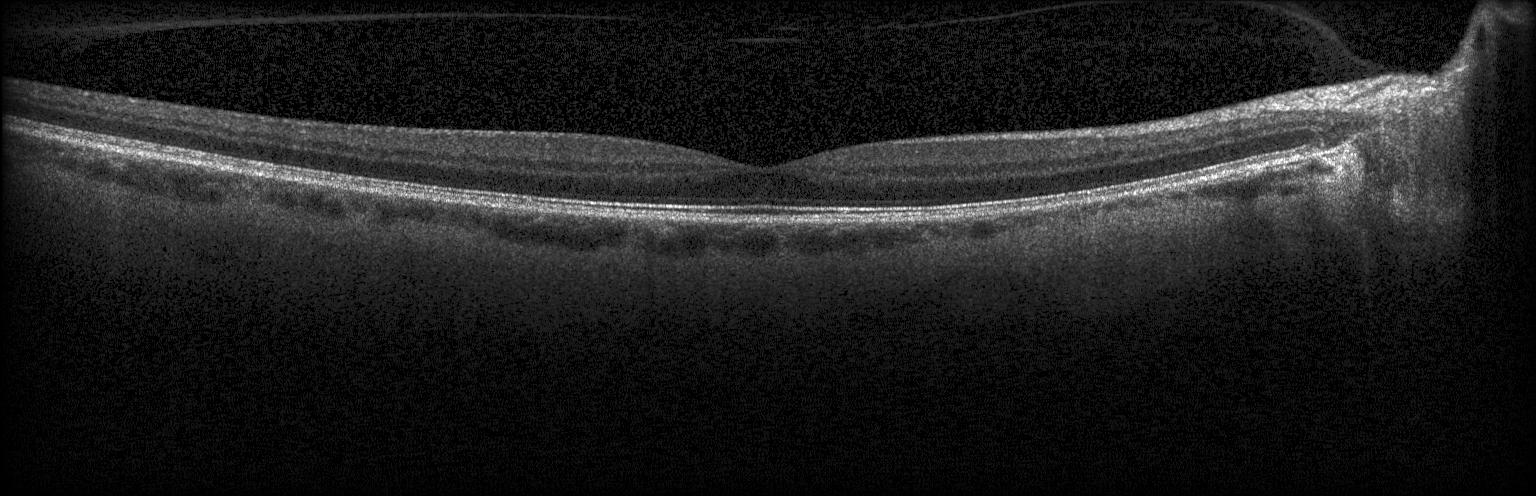 Horizontal scan through the fovea · optical coherence tomography B-scan
Diagnosis: neither choroidal neovascularization, diabetic macular edema, nor drusen.